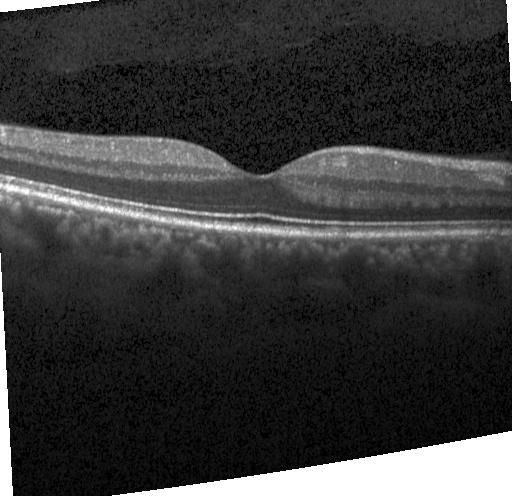 Optical coherence tomography B-scan, macular scan, spectral-domain optical coherence tomography
Assessment: no choroidal neovascularization, no diabetic macular edema, and no drusen.